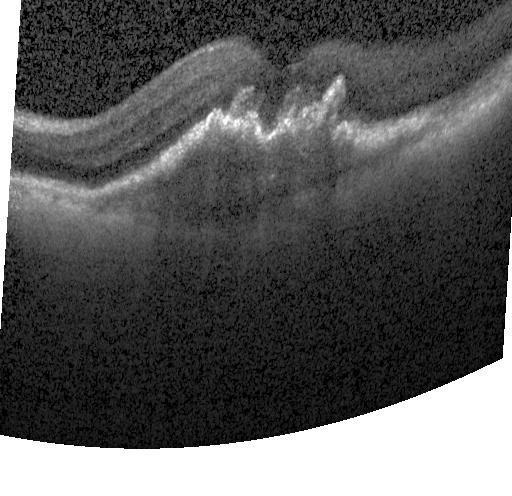 Retinal OCT cross-section.
Diagnosis: a choroidal neovascular membrane.